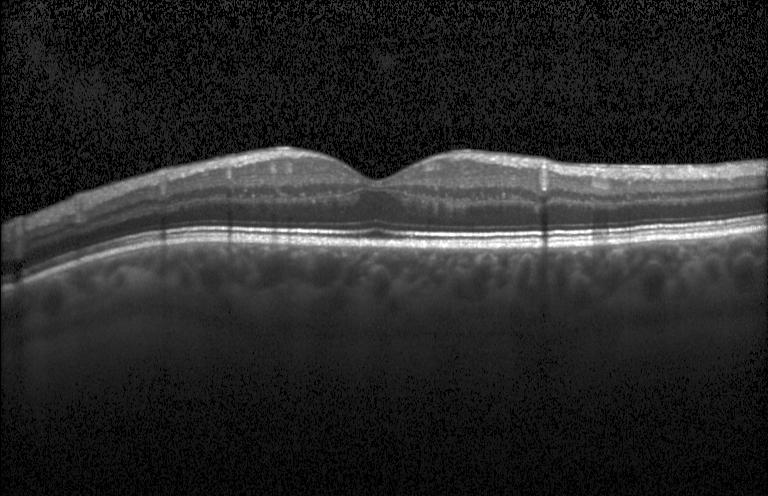
Impression: no evidence of CNV, DME, or drusen.